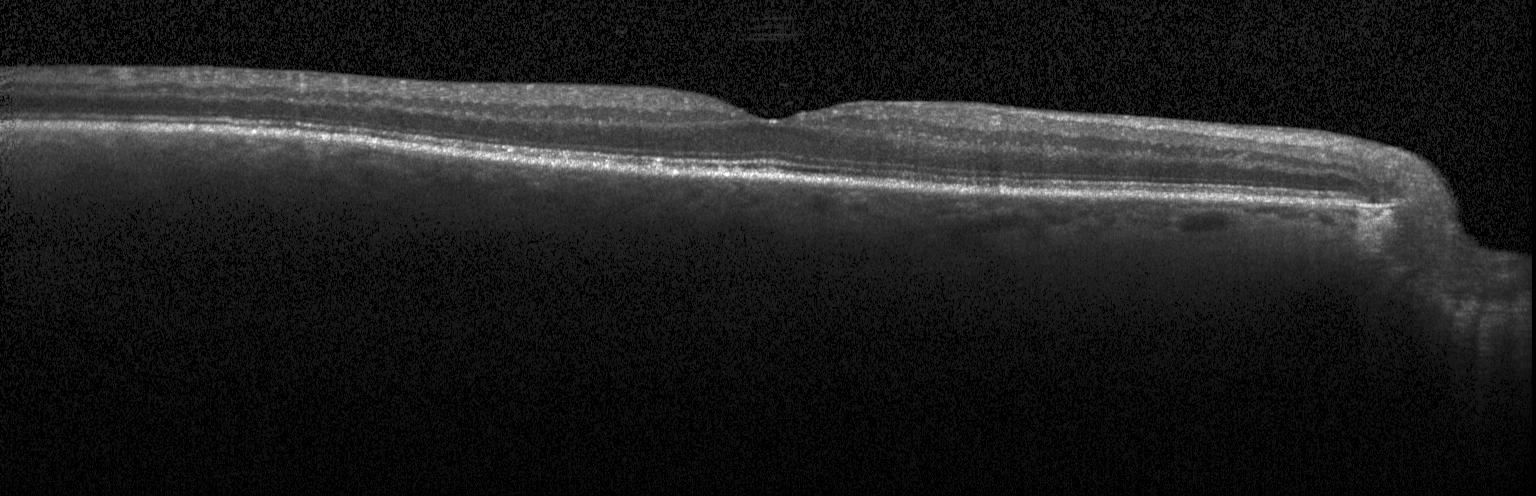

Acquired on a Heidelberg Spectralis. Optical coherence tomography B-scan — The scan shows neither choroidal neovascularization, diabetic macular edema, nor drusen.